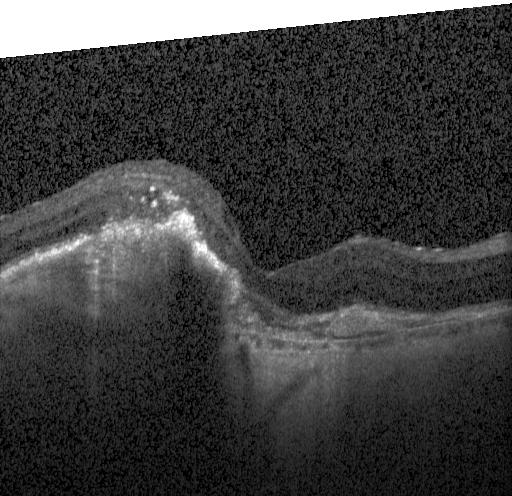
Instrument: Heidelberg Spectralis · through the macula · optical coherence tomography scan
Finding: a choroidal neovascular membrane.